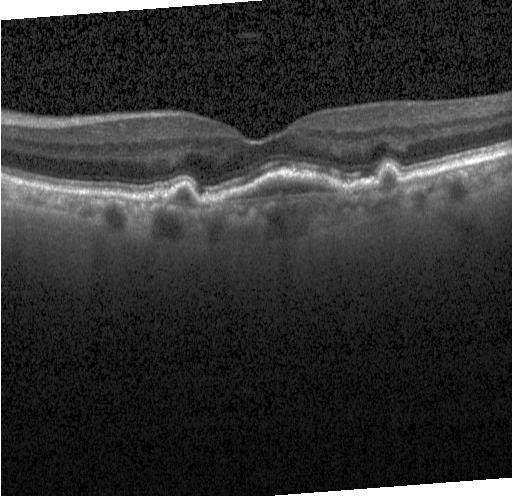
Retinal OCT B-scan; SD-OCT; centered on the fovea; acquired on a Heidelberg Spectralis.
Diagnosis: a choroidal neovascular membrane.